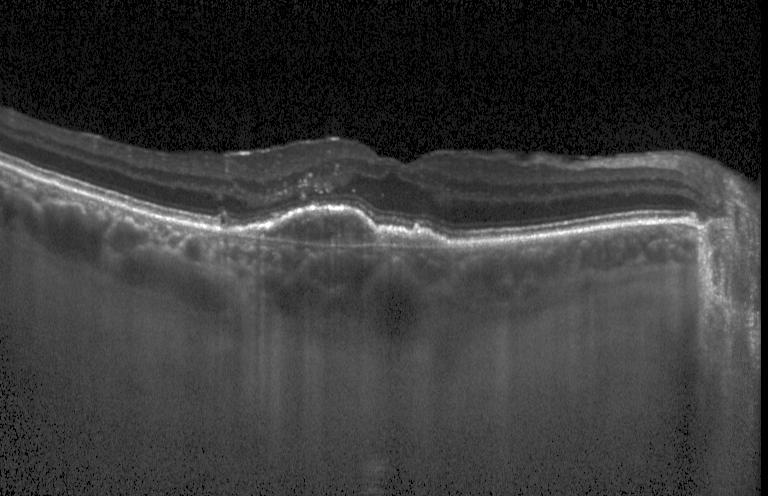
Macular OCT demonstrating choroidal neovascularization.